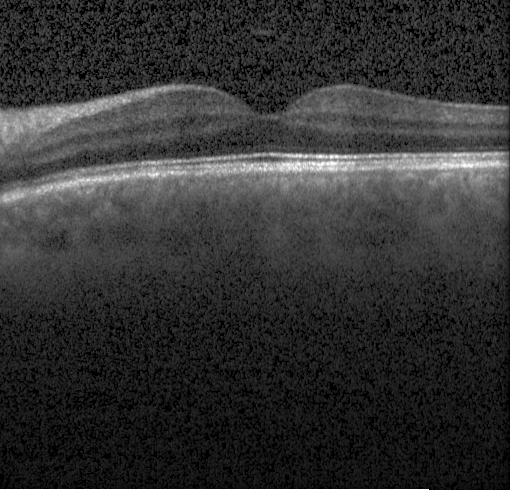
Retinal OCT B-scan — Finding: no choroidal neovascularization, diabetic macular edema, or drusen.